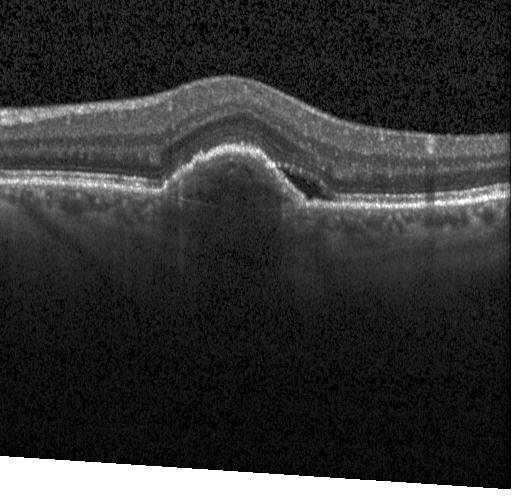 Dx: a choroidal neovascular membrane.